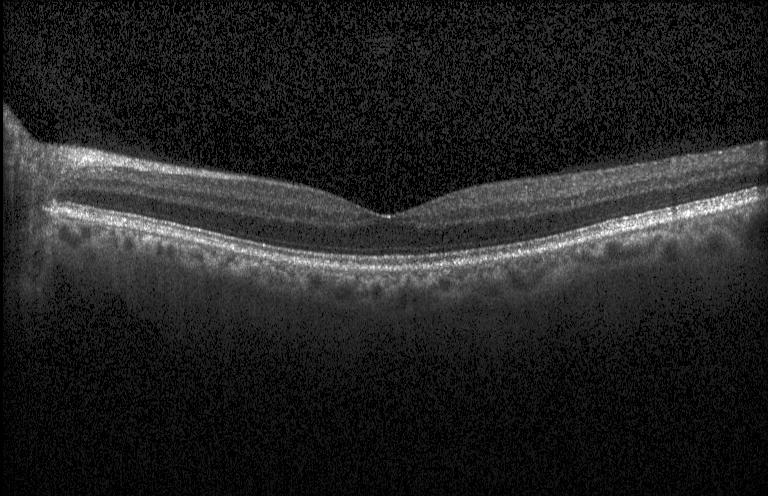

OCT B-scan; spectral-domain OCT; Heidelberg Spectralis; centered on the fovea. No CNV, no DME, and no drusen.